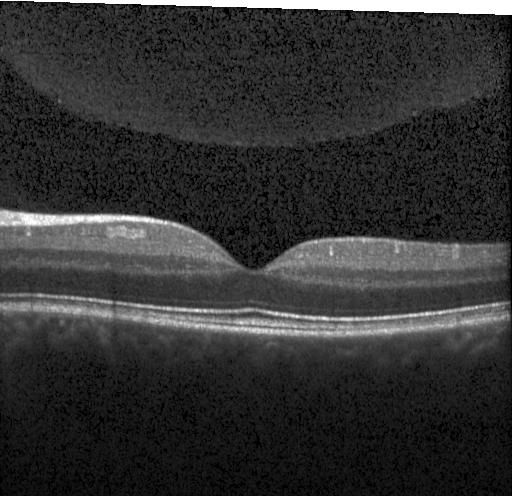
Optical coherence tomography B-scan.
Finding: neither choroidal neovascularization, diabetic macular edema, nor drusen.